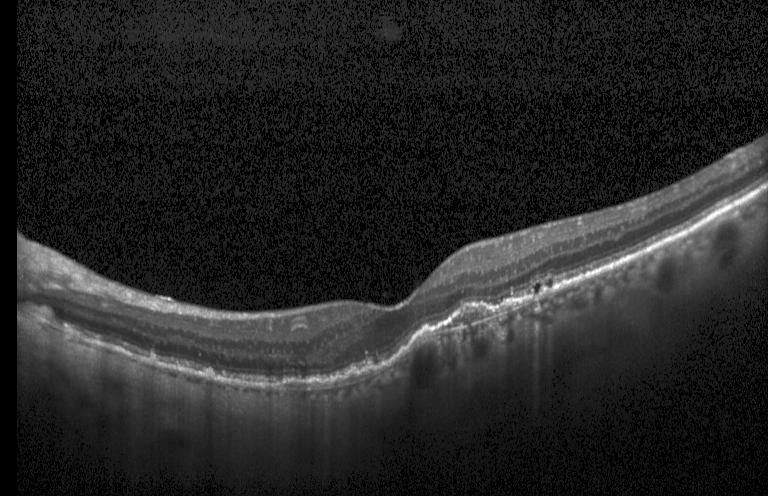
Diagnosis: CNV.